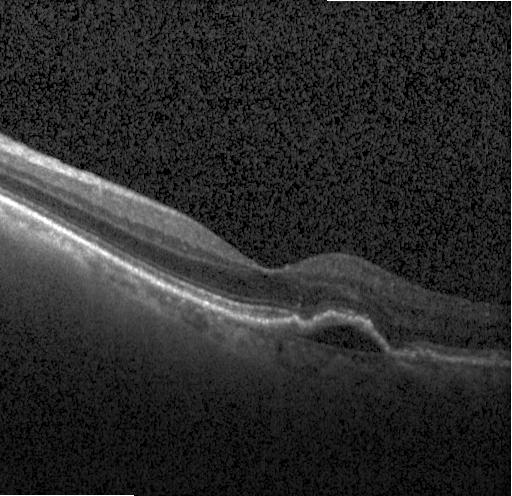

Spectral-domain OCT · optical coherence tomography scan. Impression: a choroidal neovascular membrane.